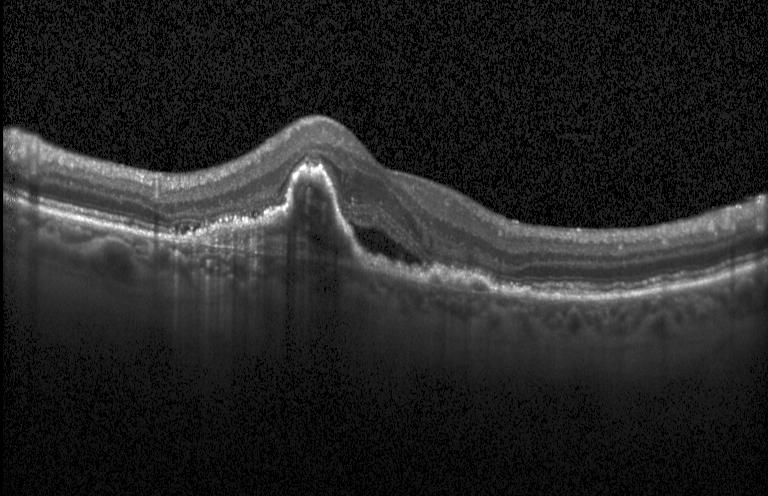

Macular scan, retinal OCT B-scan, instrument: Heidelberg Spectralis. Diagnosis: a choroidal neovascular membrane.